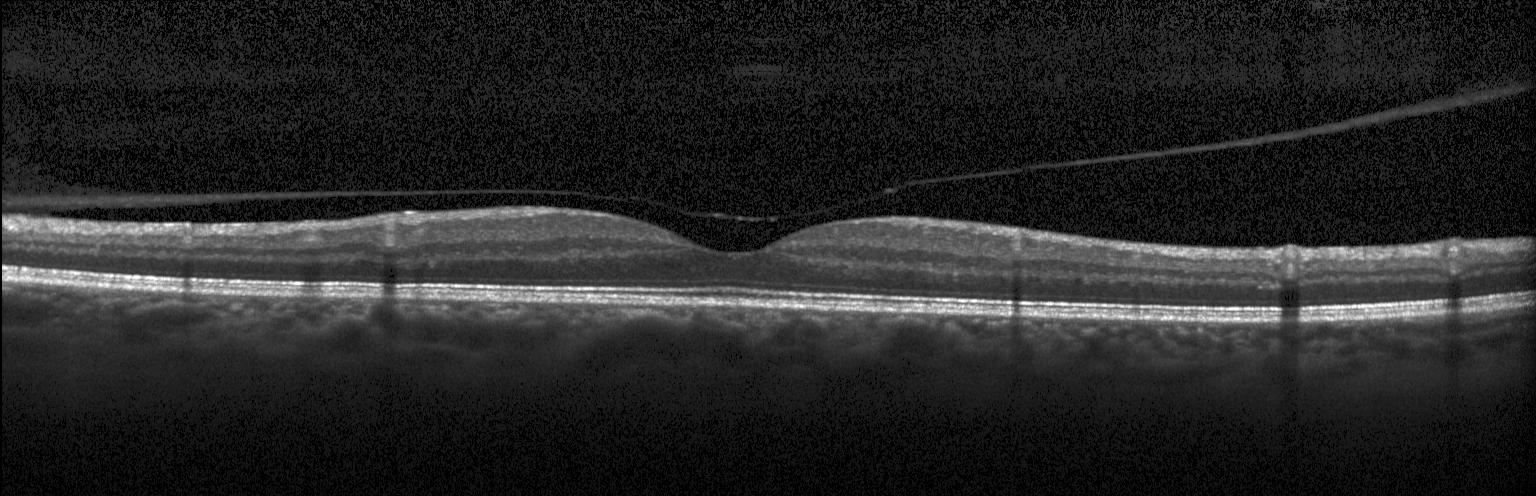
Fovea-centered. Spectral-domain OCT. OCT line scan. Heidelberg Spectralis. OCT finding: no CNV, DME, or drusen.